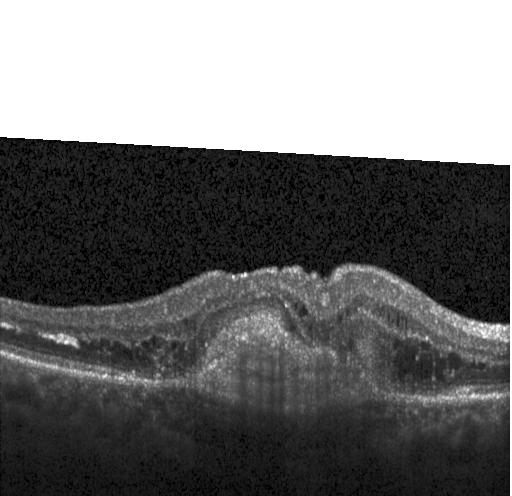
Retinal OCT B-scan. Instrument: Heidelberg Spectralis — A choroidal neovascular membrane.